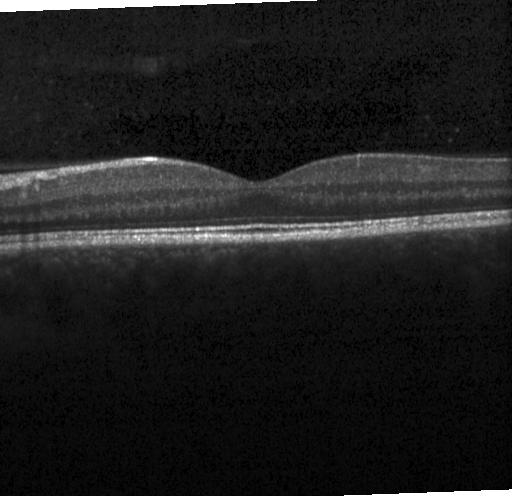 Optical coherence tomography B-scan · spectral-domain optical coherence tomography — Assessment: no CNV, no DME, and no drusen.